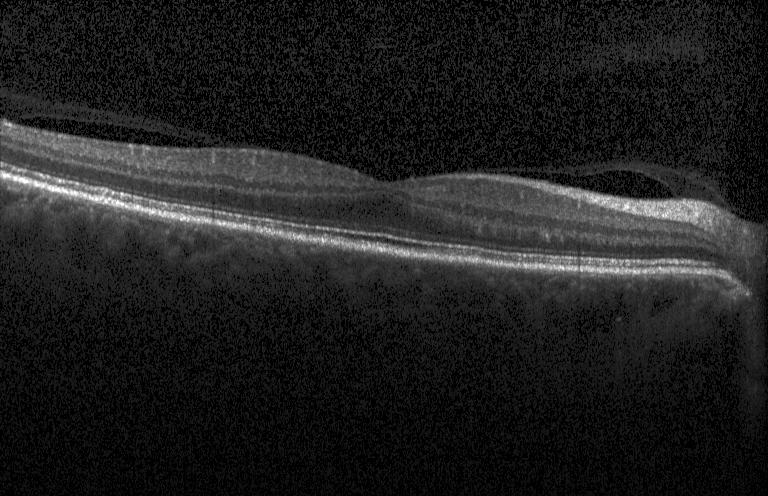
Diagnosis: no evidence of CNV, DME, or drusen.